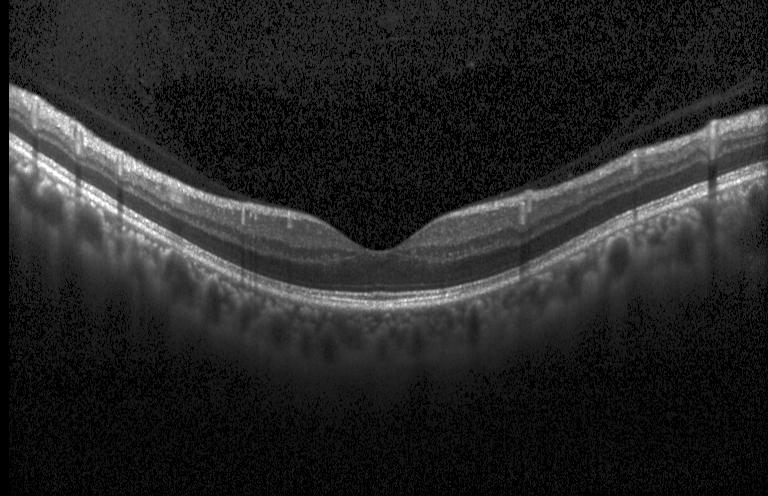

Retinal OCT cross-section — Impression: no choroidal neovascularization, diabetic macular edema, or drusen.